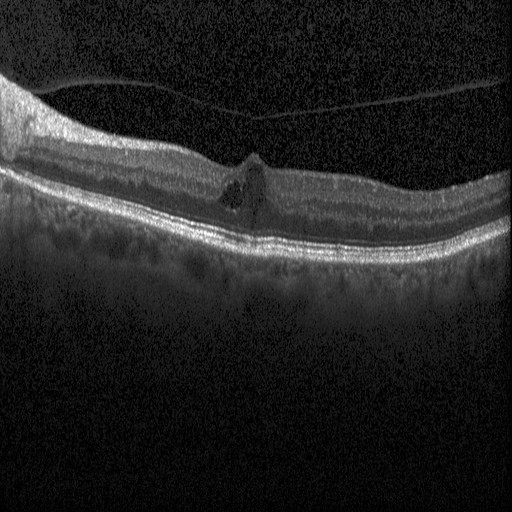 Macular OCT demonstrating DME.